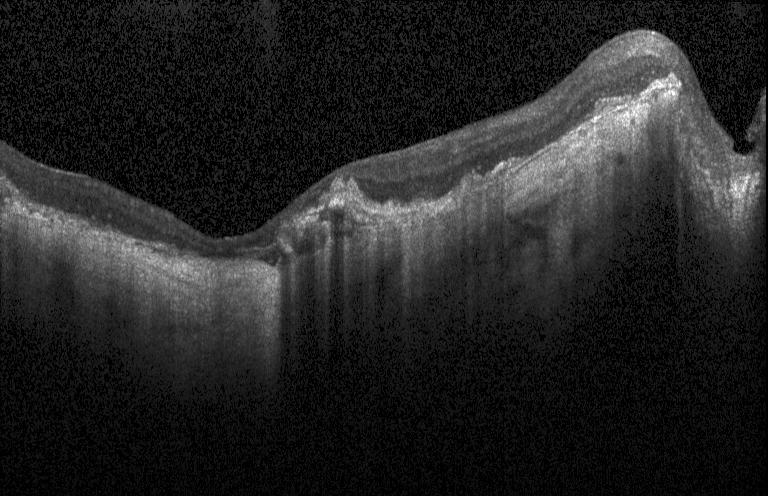 Optical coherence tomography scan.
OCT finding: choroidal neovascularization (CNV).